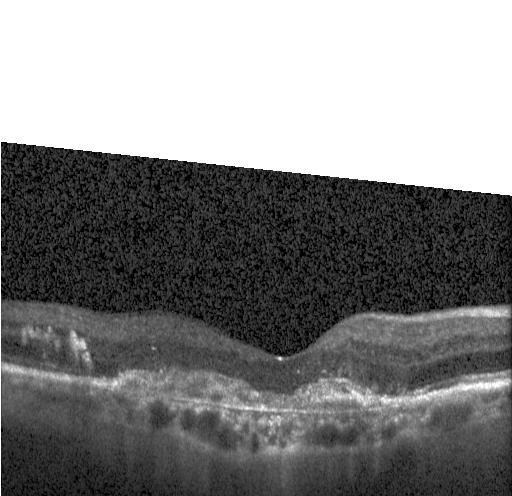
Through the macula. Spectral-domain OCT. Retinal OCT B-scan — Assessment: a choroidal neovascular membrane.